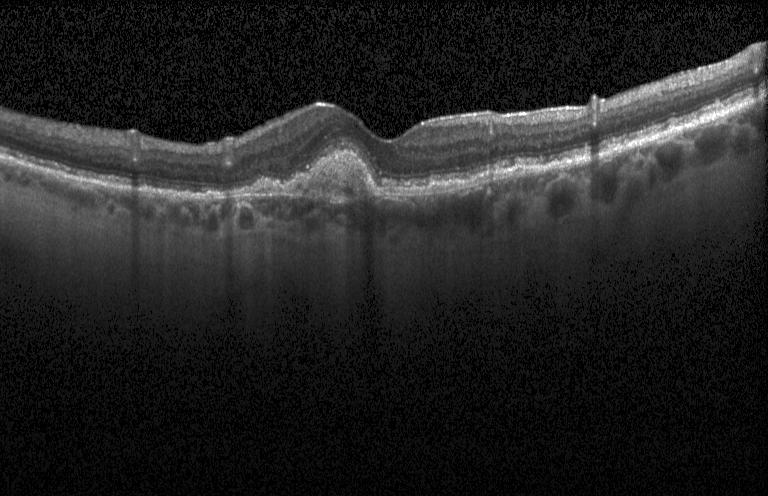 Horizontal scan through the fovea · retinal OCT cross-section · Heidelberg Spectralis · spectral-domain optical coherence tomography
This B-scan demonstrates choroidal neovascularization.